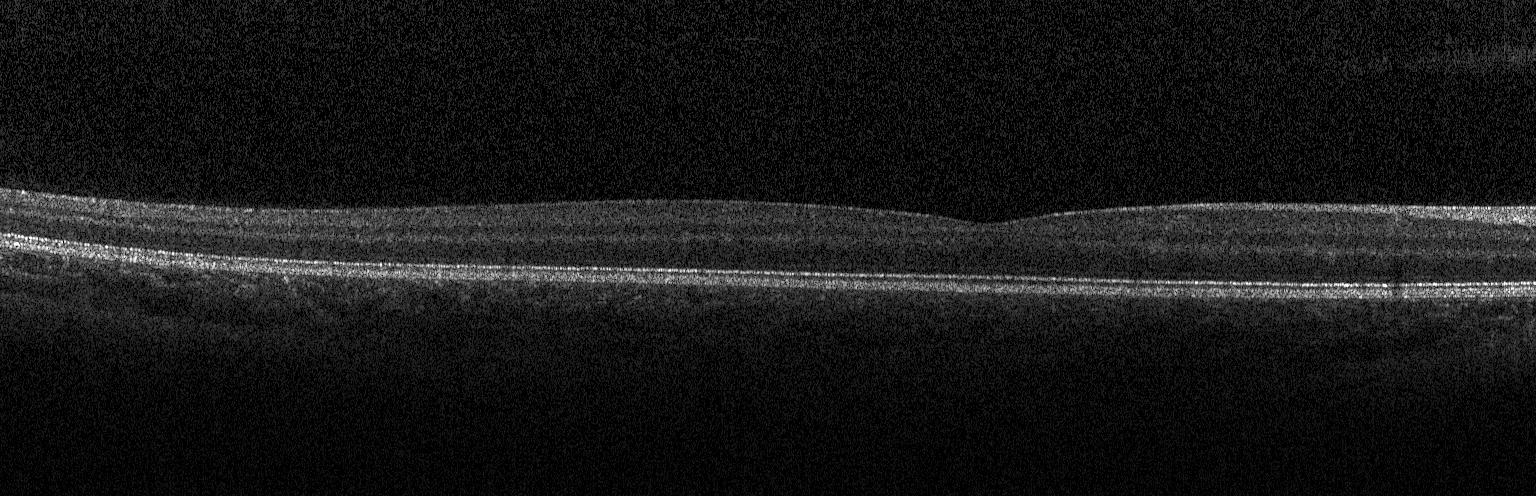
Optical coherence tomography scan; Heidelberg Spectralis; SD-OCT; centered on the fovea. Impression: no choroidal neovascularization, diabetic macular edema, or drusen.